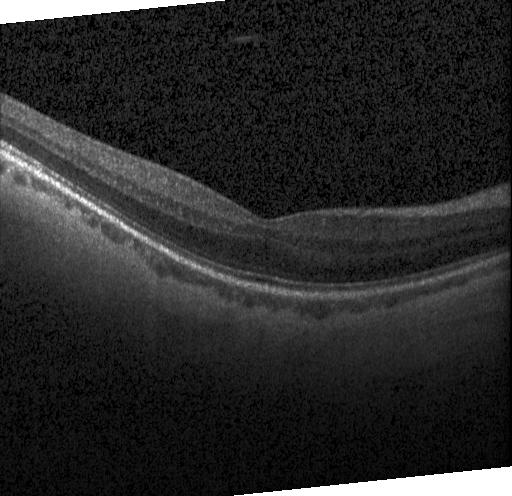
Optical coherence tomography scan; acquired on a Heidelberg Spectralis — Finding: neither CNV, DME, nor drusen.